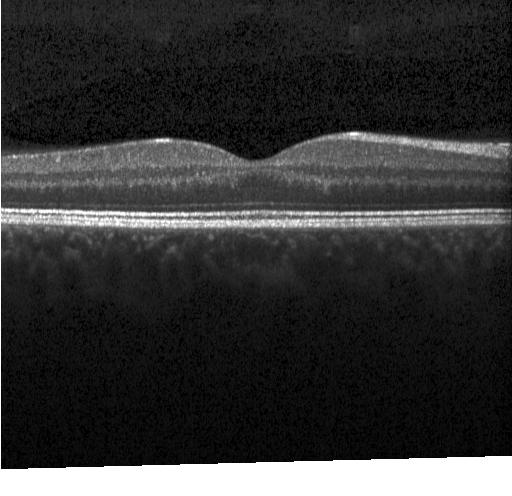

Dx: no choroidal neovascularization, no diabetic macular edema, and no drusen.